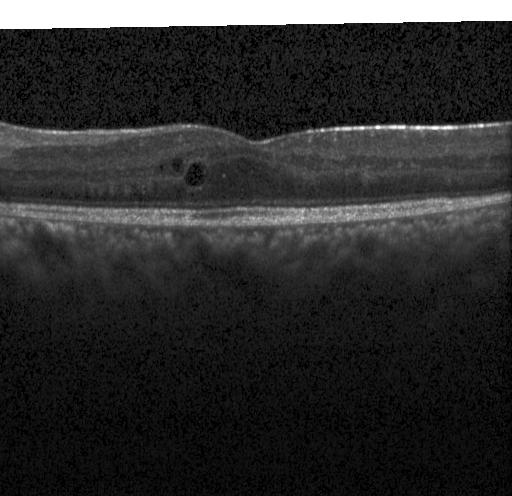

Diagnosis: DME.